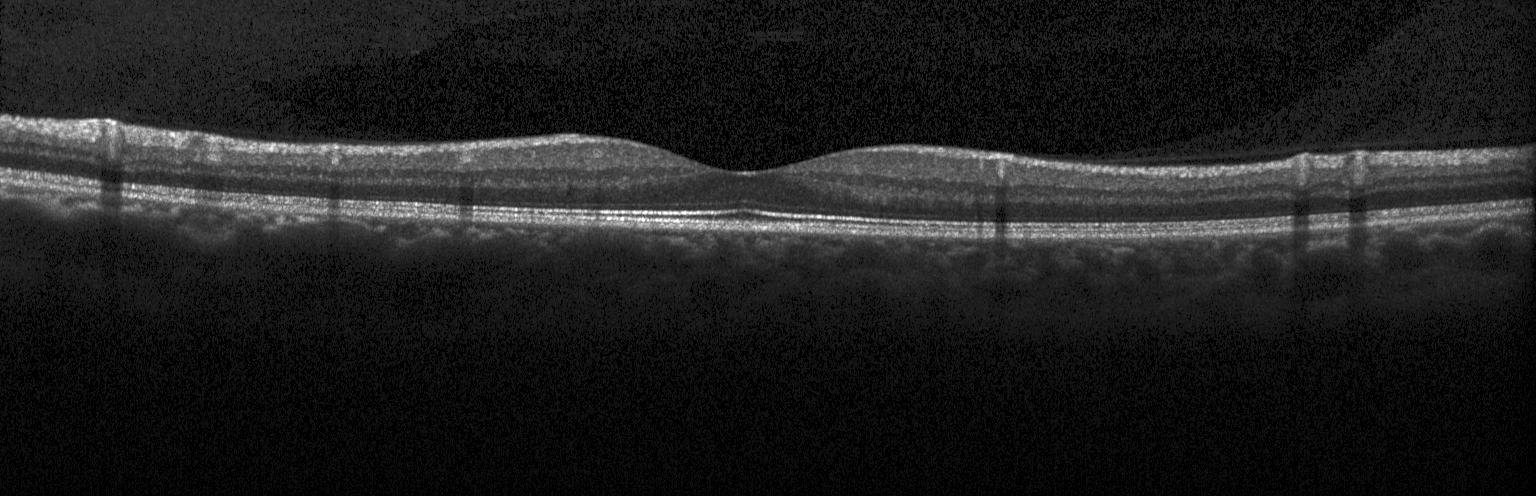 Impression: no choroidal neovascularization, diabetic macular edema, or drusen.